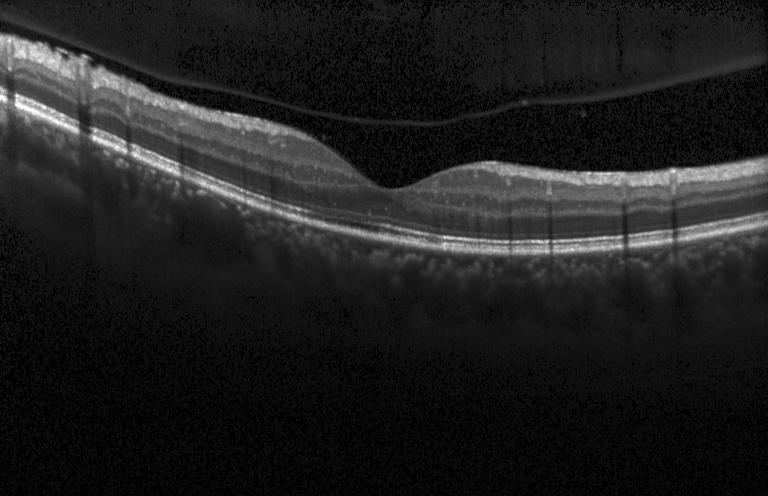 Optical coherence tomography scan — Macular OCT: no choroidal neovascularization, no diabetic macular edema, and no drusen.